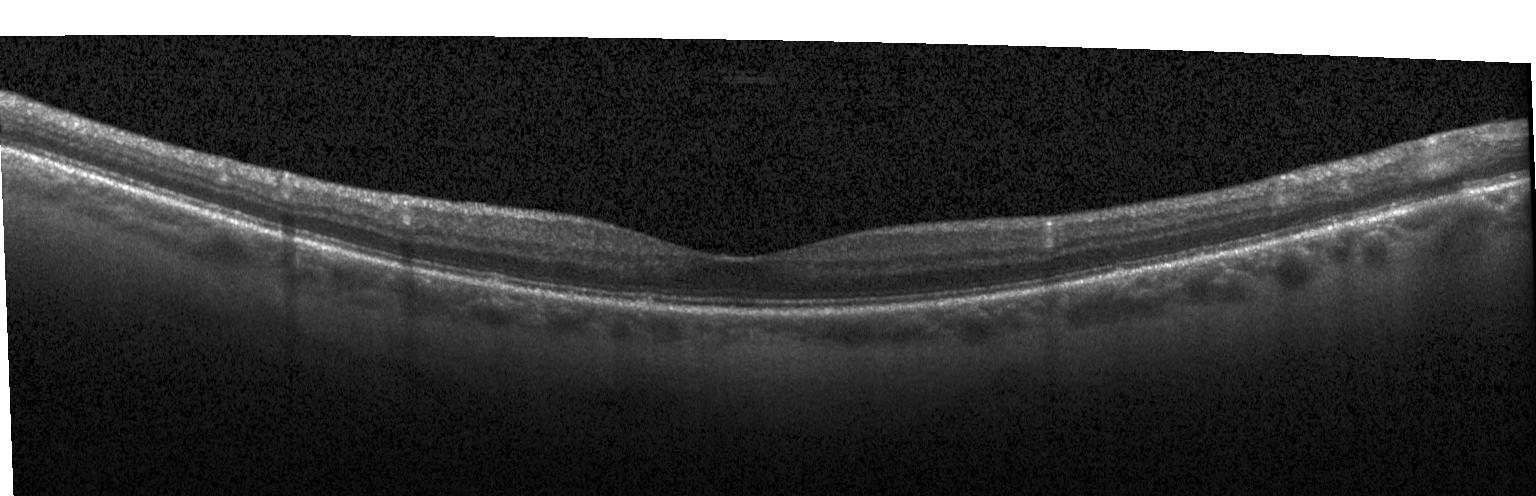

OCT line scan. SD-OCT. Fovea-centered
Macular OCT: neither CNV, DME, nor drusen.